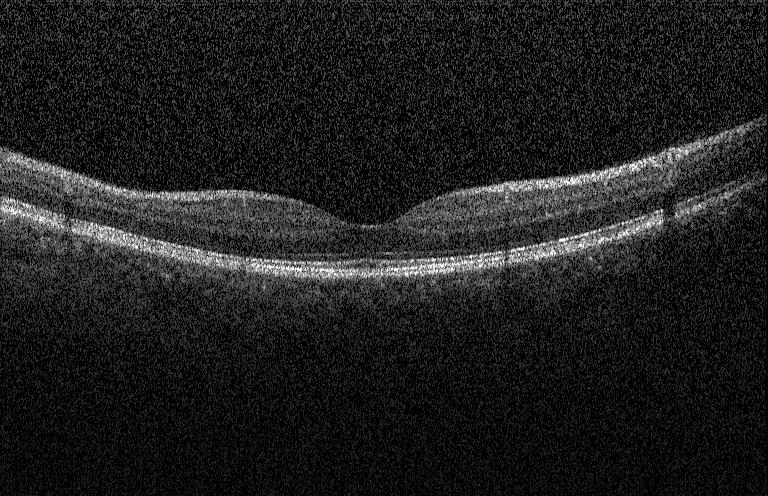
Spectral-domain OCT · OCT B-scan · centered on the fovea — OCT finding: no choroidal neovascularization, diabetic macular edema, or drusen.